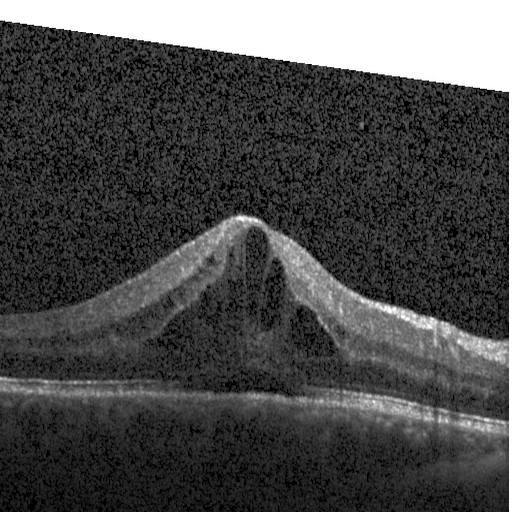

Heidelberg Spectralis; optical coherence tomography scan. The scan shows DME.